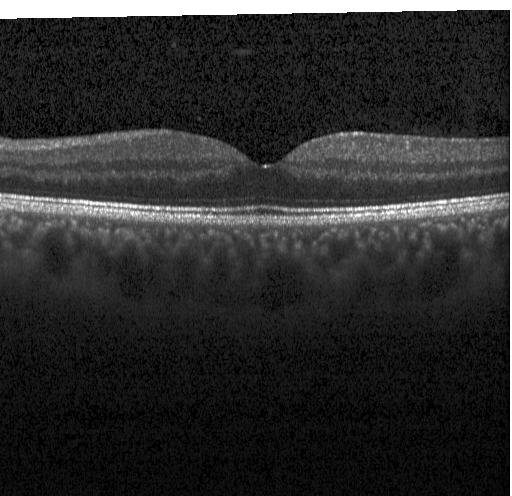 Retinal OCT cross-section
Impression: no CNV, DME, or drusen.